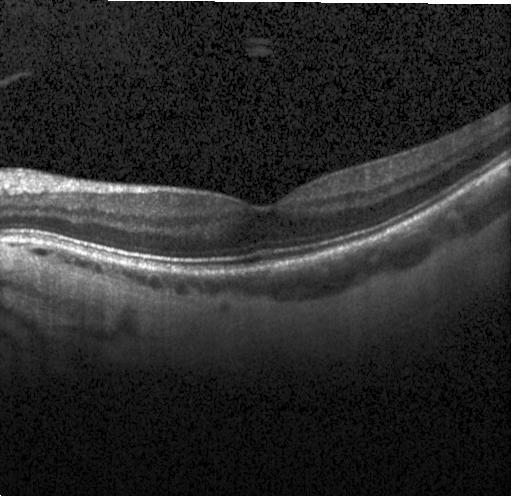
Spectral-domain optical coherence tomography; optical coherence tomography B-scan — The scan shows no CNV, DME, or drusen.